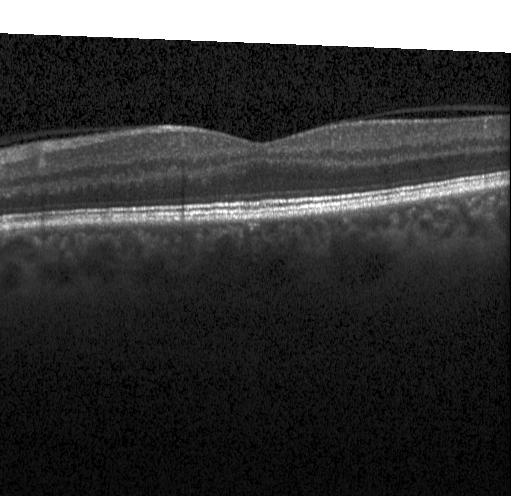

SD-OCT, optical coherence tomography scan, centered on the fovea. Macular OCT: neither choroidal neovascularization, diabetic macular edema, nor drusen.